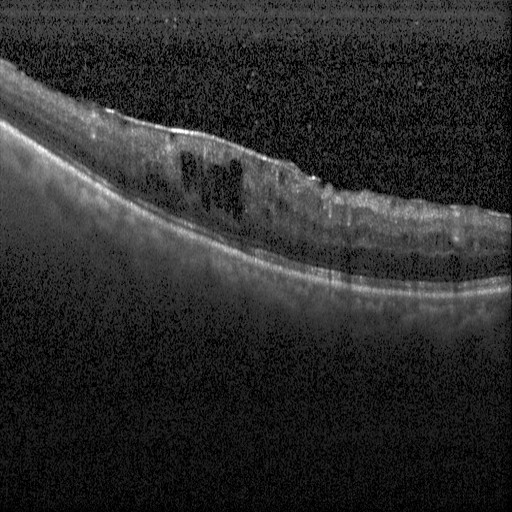 SD-OCT · OCT B-scan — Assessment: diabetic macular edema.